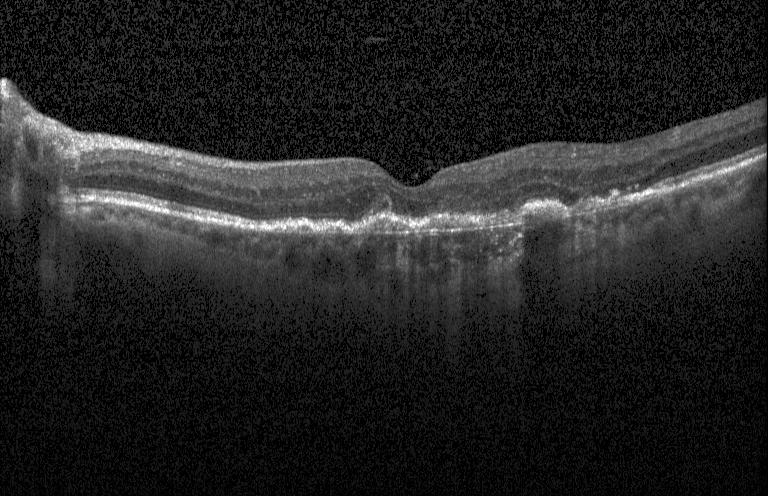

Heidelberg Spectralis · optical coherence tomography B-scan · through the macula · SD-OCT.
This B-scan demonstrates choroidal neovascularization.